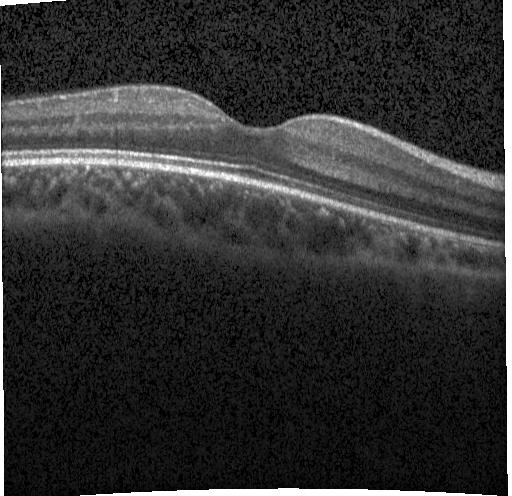

Optical coherence tomography scan, fovea-centered, spectral-domain optical coherence tomography, acquired on a Heidelberg Spectralis — Impression: no choroidal neovascularization, no diabetic macular edema, and no drusen.